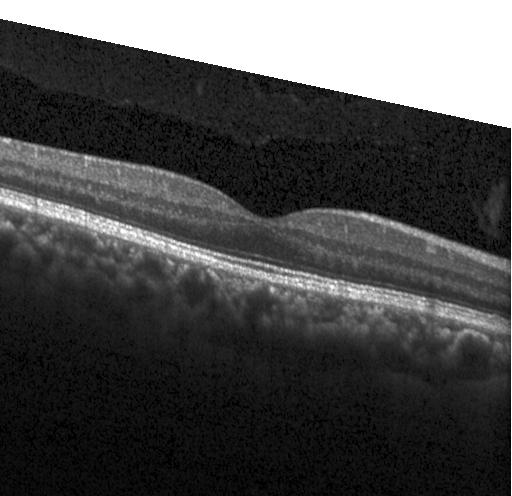
Acquired on a Heidelberg Spectralis, through the macula, retinal OCT cross-section, spectral-domain OCT.
Macular OCT: no choroidal neovascularization, no diabetic macular edema, and no drusen.